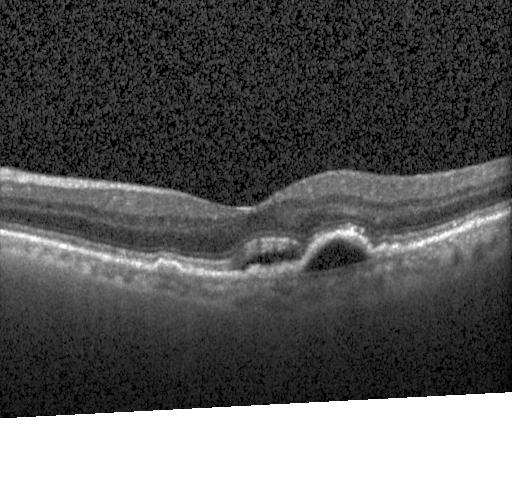

Acquired on a Heidelberg Spectralis, optical coherence tomography B-scan, spectral-domain optical coherence tomography
Dx: choroidal neovascularization.